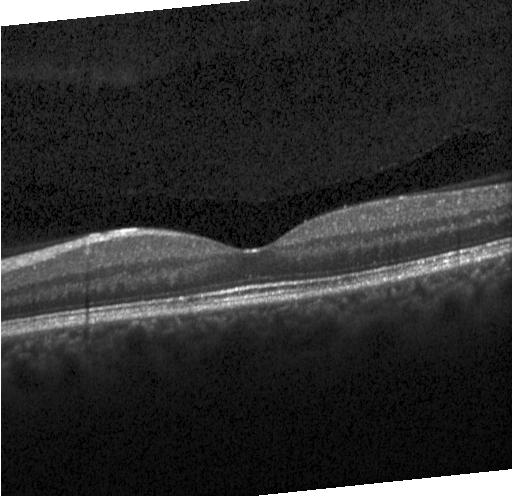 Optical coherence tomography scan, spectral-domain OCT
Assessment: neither choroidal neovascularization, diabetic macular edema, nor drusen.